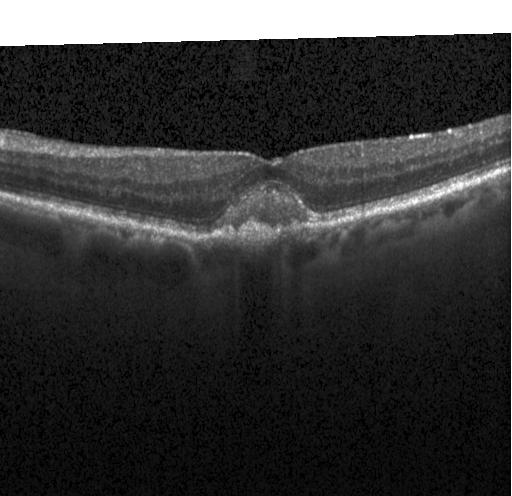 This B-scan demonstrates a choroidal neovascular membrane.